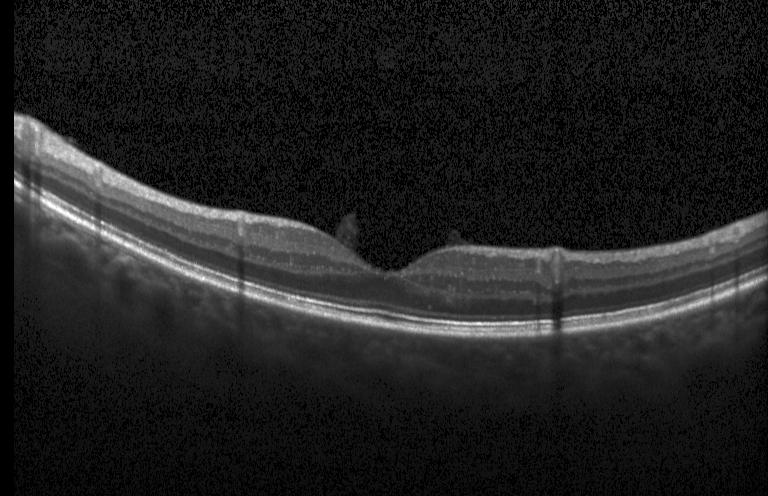
Spectral-domain optical coherence tomography. Retinal OCT B-scan. Acquired on a Heidelberg Spectralis.
Diagnosis: no CNV, DME, or drusen.